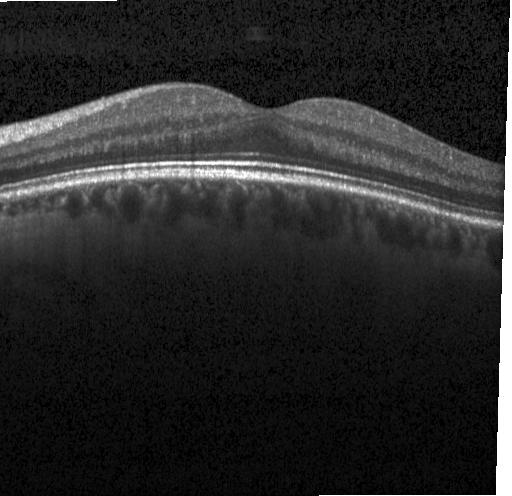
Diagnosis: neither CNV, DME, nor drusen.